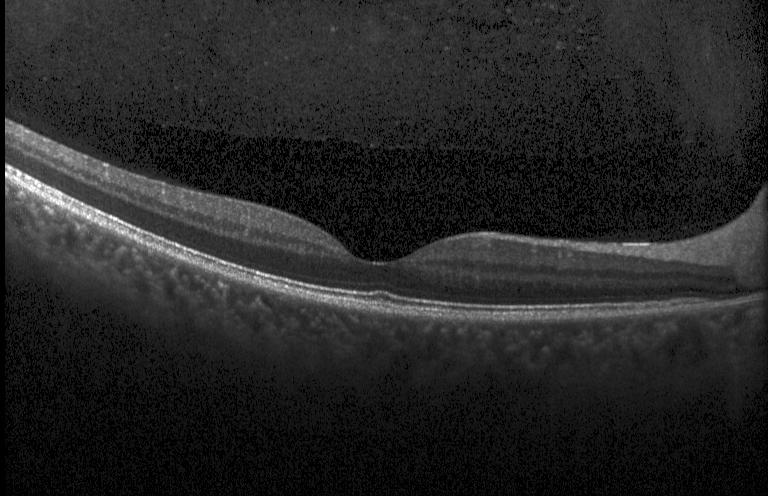 Diagnosis: no choroidal neovascularization, no diabetic macular edema, and no drusen.